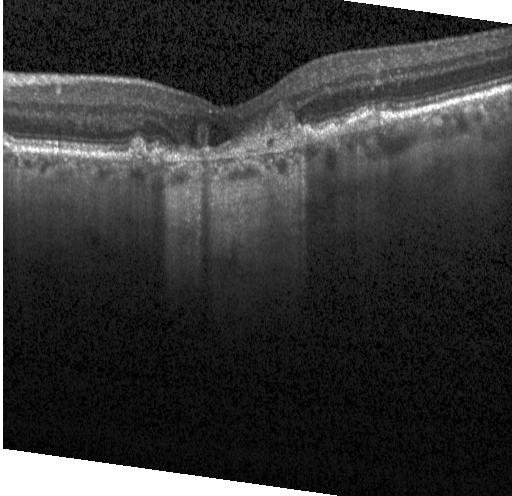

Through the macula. OCT B-scan. Acquired on a Heidelberg Spectralis
Choroidal neovascularization (CNV).